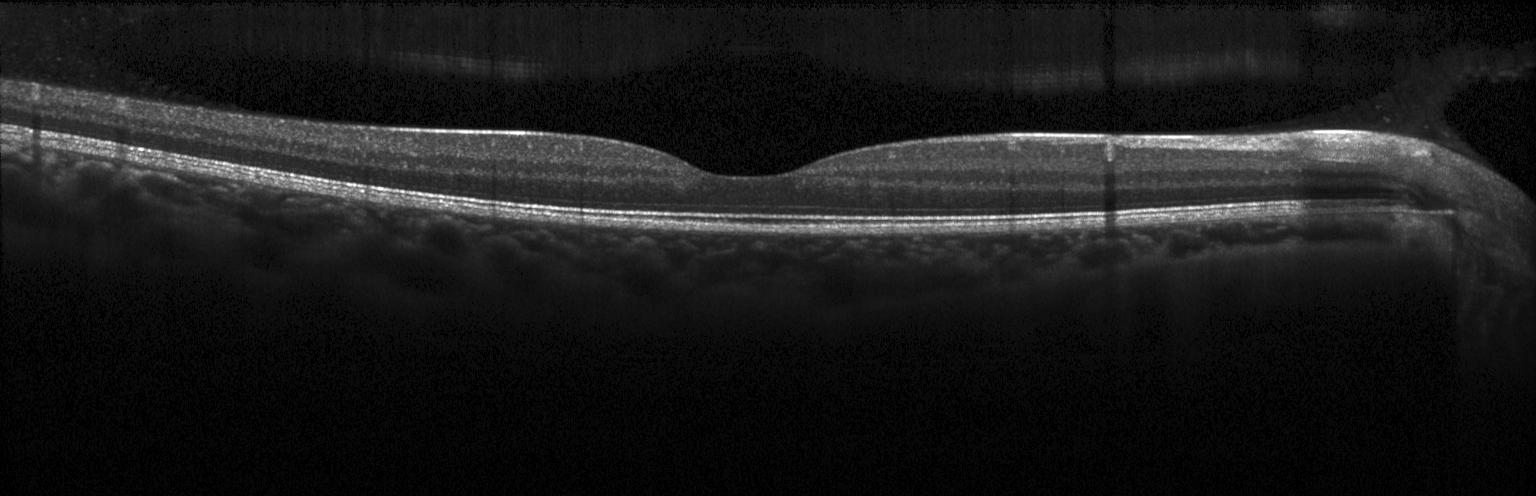
Retinal OCT cross-section. Through the macula.
Diagnosis: no CNV, DME, or drusen.